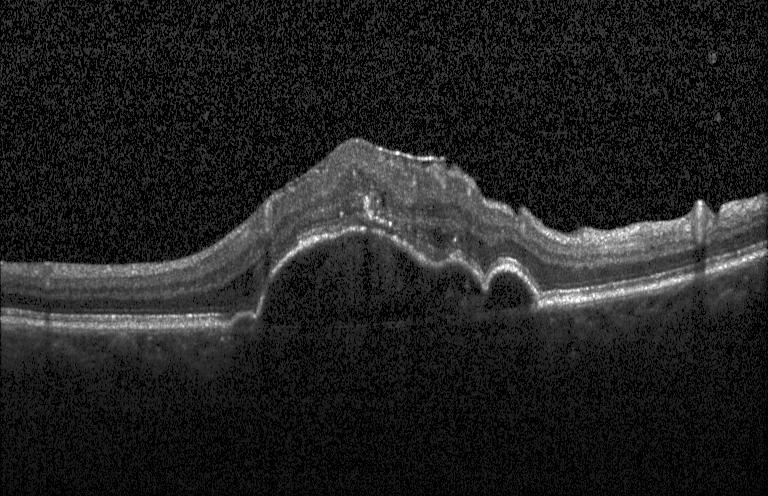 Retinal OCT cross-section showing a choroidal neovascular membrane.